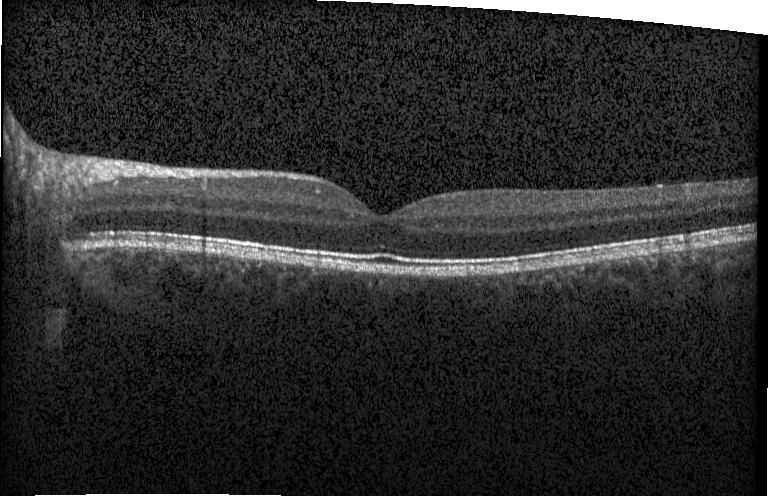 Impression: neither choroidal neovascularization, diabetic macular edema, nor drusen.